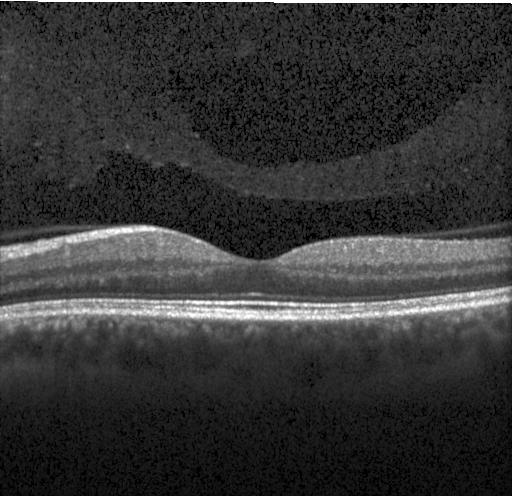
OCT finding: no evidence of choroidal neovascularization, diabetic macular edema, or drusen.